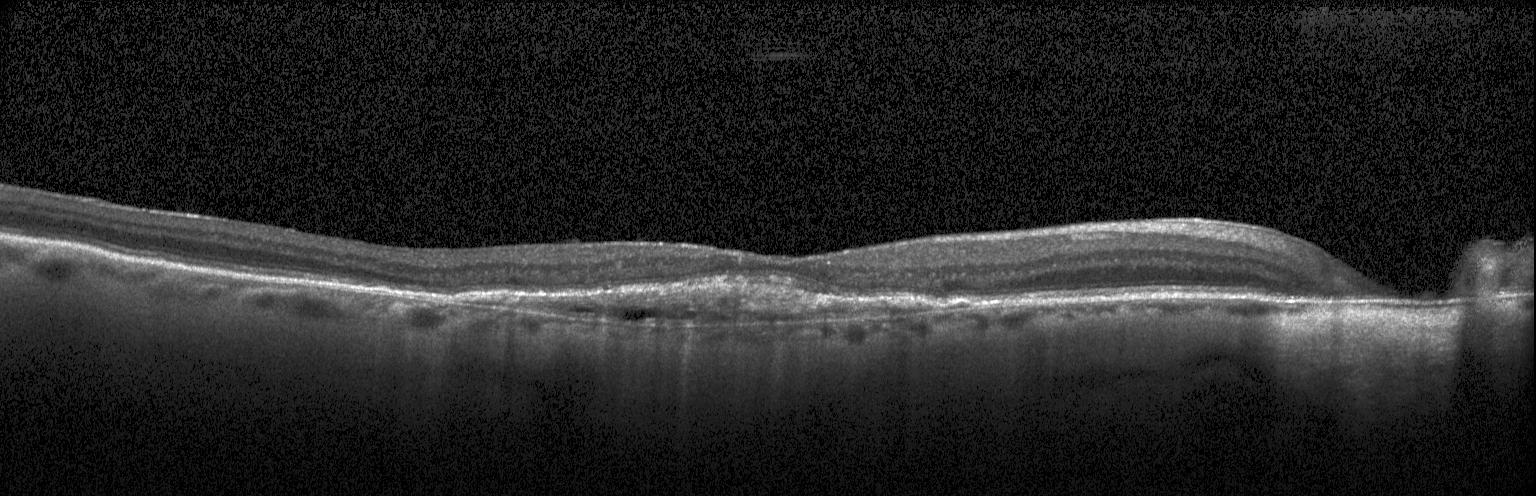 Macular scan. Optical coherence tomography B-scan. Spectral-domain optical coherence tomography. Heidelberg Spectralis. Finding: a choroidal neovascular membrane.